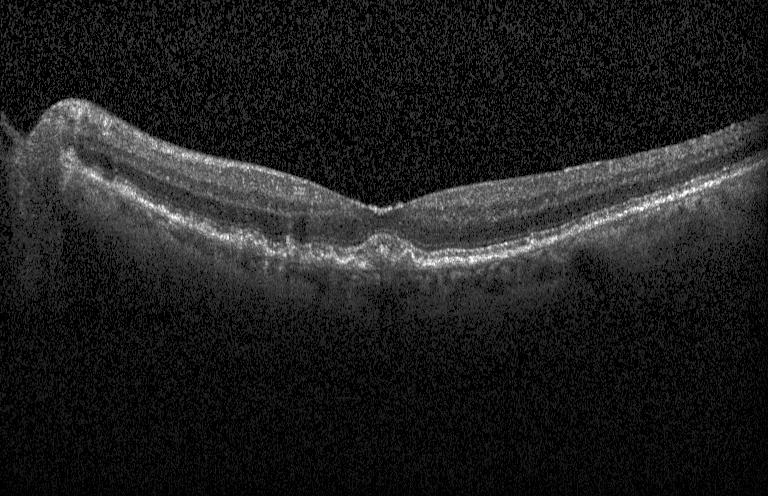
Optical coherence tomography B-scan. Assessment: drusen.